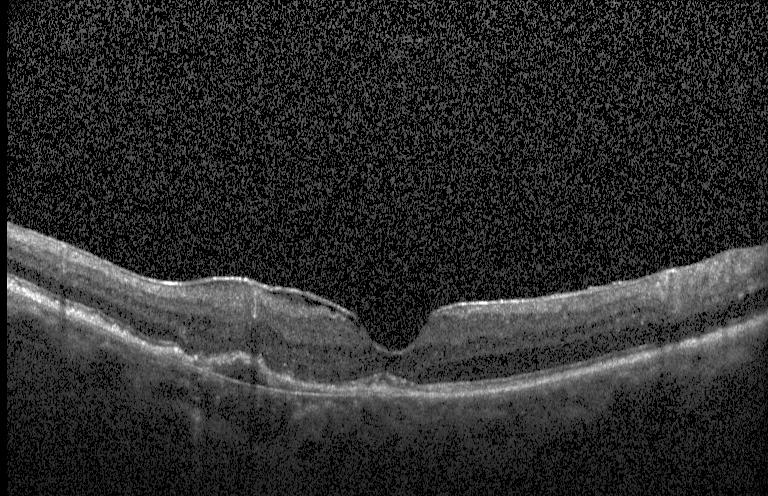 Retinal OCT cross-section. Diagnosis: a choroidal neovascular membrane.